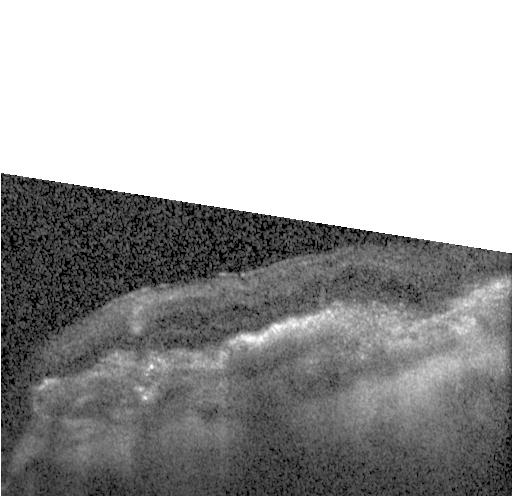 Heidelberg Spectralis, retinal OCT B-scan. Dx: a choroidal neovascular membrane.